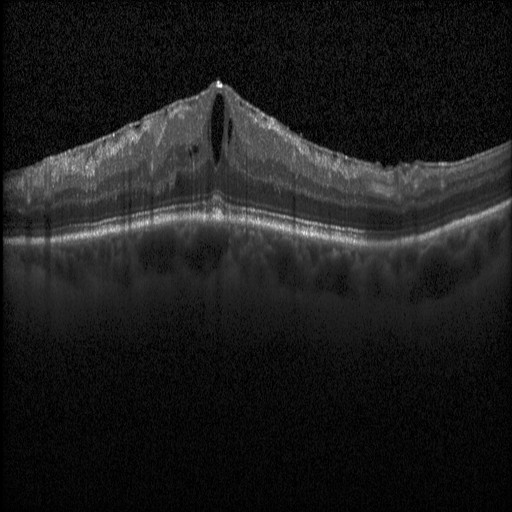 Finding: diabetic macular edema.